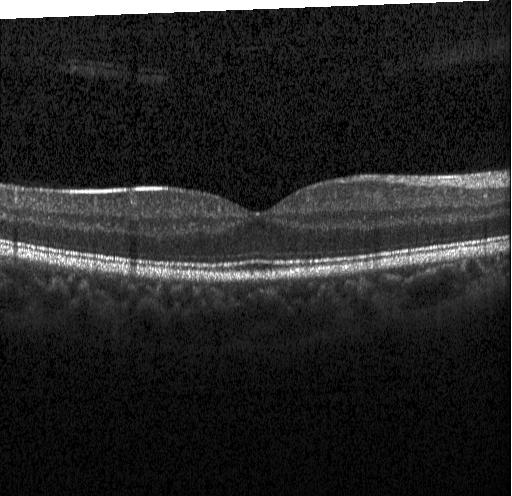
Dx: neither CNV, DME, nor drusen.